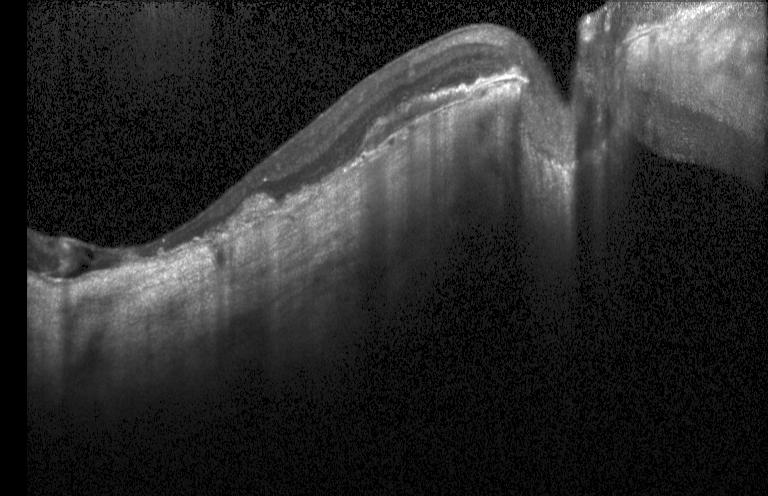

OCT line scan, spectral-domain OCT, Heidelberg Spectralis, macular scan.
Impression: choroidal neovascularization (CNV).